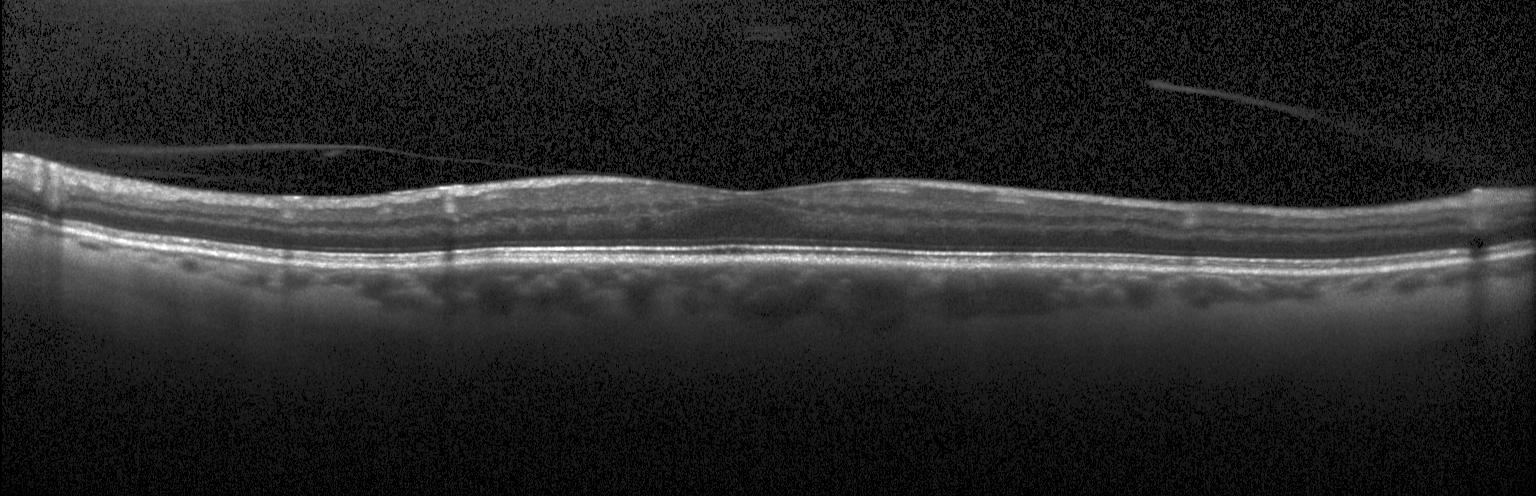
Finding: neither choroidal neovascularization, diabetic macular edema, nor drusen.